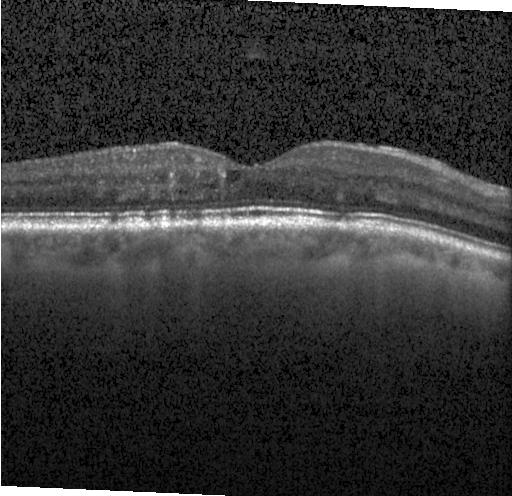
Optical coherence tomography B-scan, spectral-domain OCT, Heidelberg Spectralis, through the macula.
The scan shows diabetic macular edema.